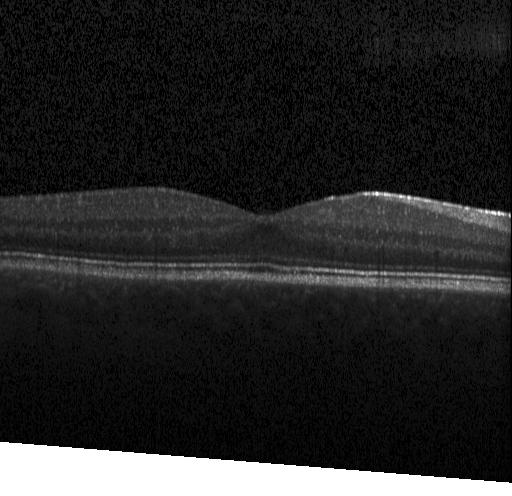

Impression: no evidence of choroidal neovascularization, diabetic macular edema, or drusen.